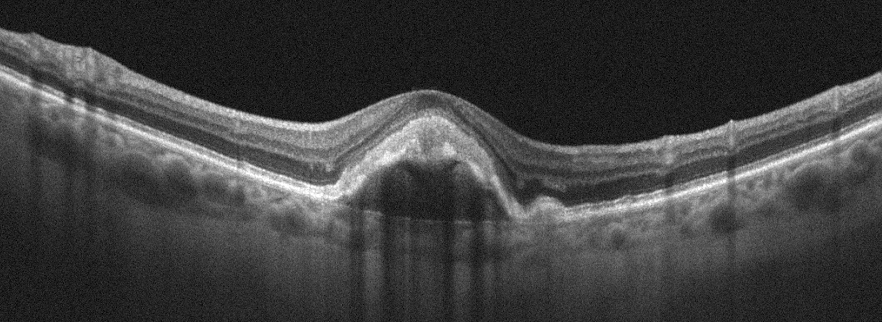
Optical coherence tomography scan
This B-scan demonstrates age-related macular degeneration.